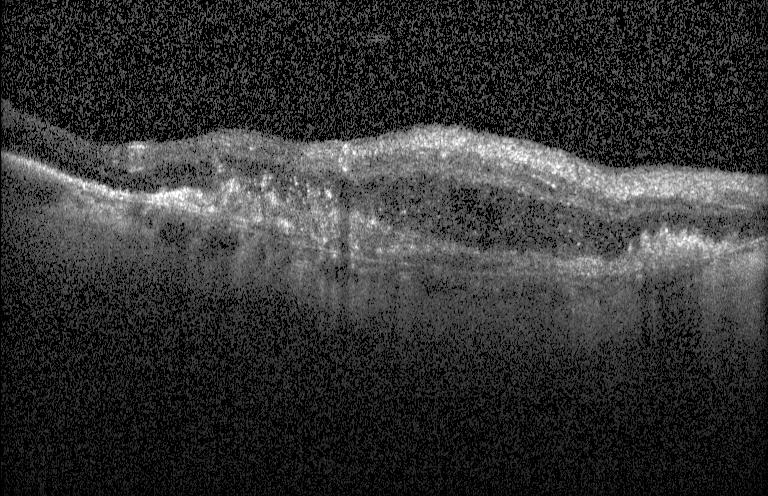
Spectral-domain optical coherence tomography; through the macula; retinal OCT cross-section; Heidelberg Spectralis — OCT finding: CNV.